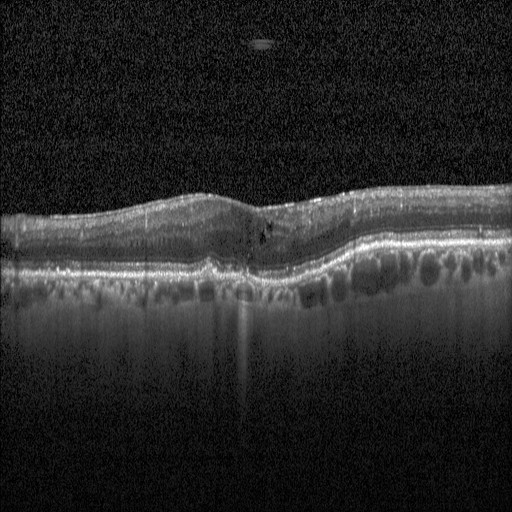

DME.